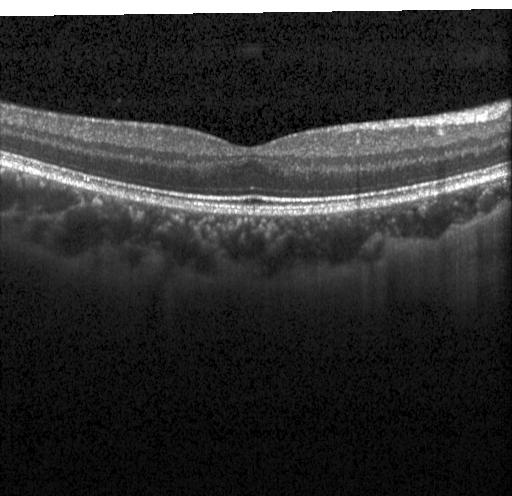 Finding: no CNV, no DME, and no drusen.